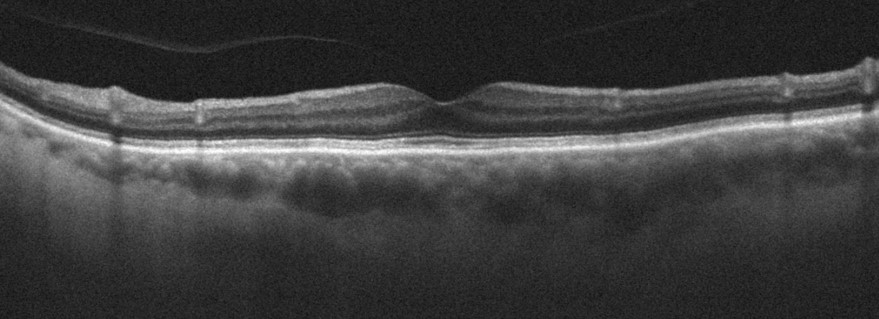 Assessment: no AMD, DME, ERM, RAO, RVO, or VID.